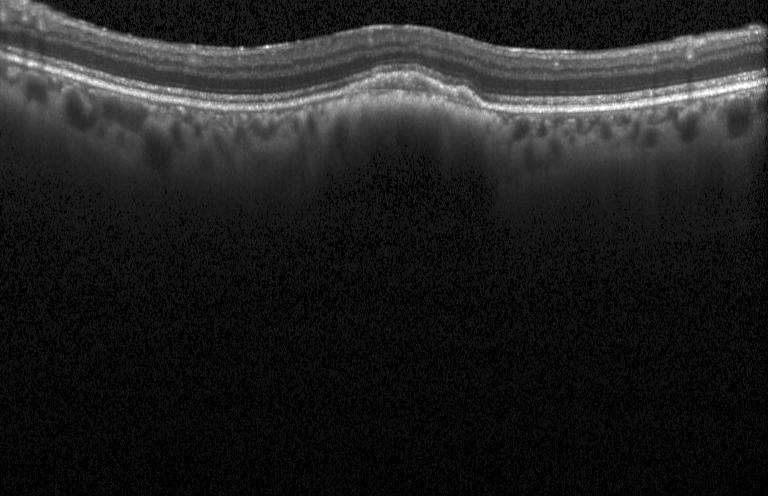 Macular scan, optical coherence tomography scan, spectral-domain OCT, Heidelberg Spectralis
Choroidal neovascularization (CNV).